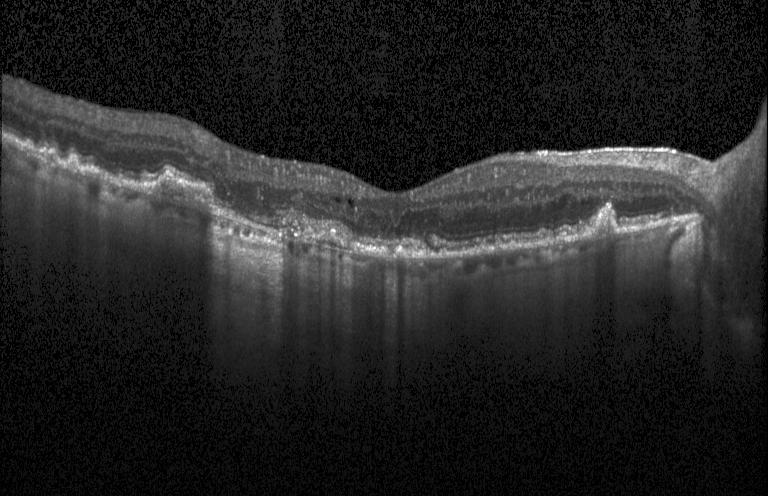

Retinal OCT B-scan
The scan shows CNV.